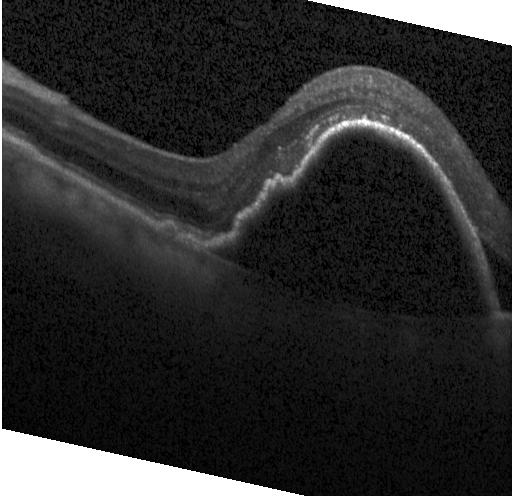

Centered on the fovea. Spectral-domain optical coherence tomography. Retinal OCT cross-section. Instrument: Heidelberg Spectralis
Choroidal neovascularization (CNV).